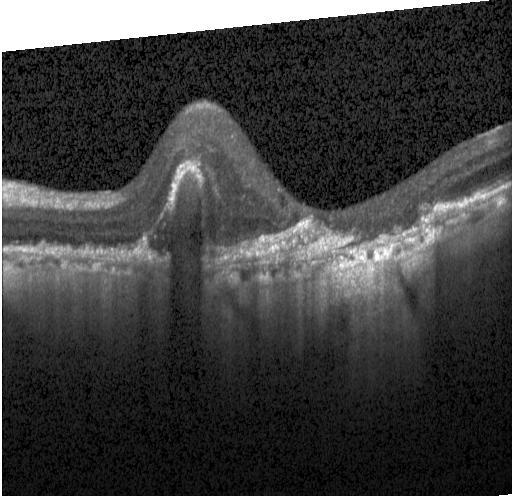
SD-OCT · optical coherence tomography B-scan · acquired on a Heidelberg Spectralis · centered on the fovea. Macular OCT: a choroidal neovascular membrane.